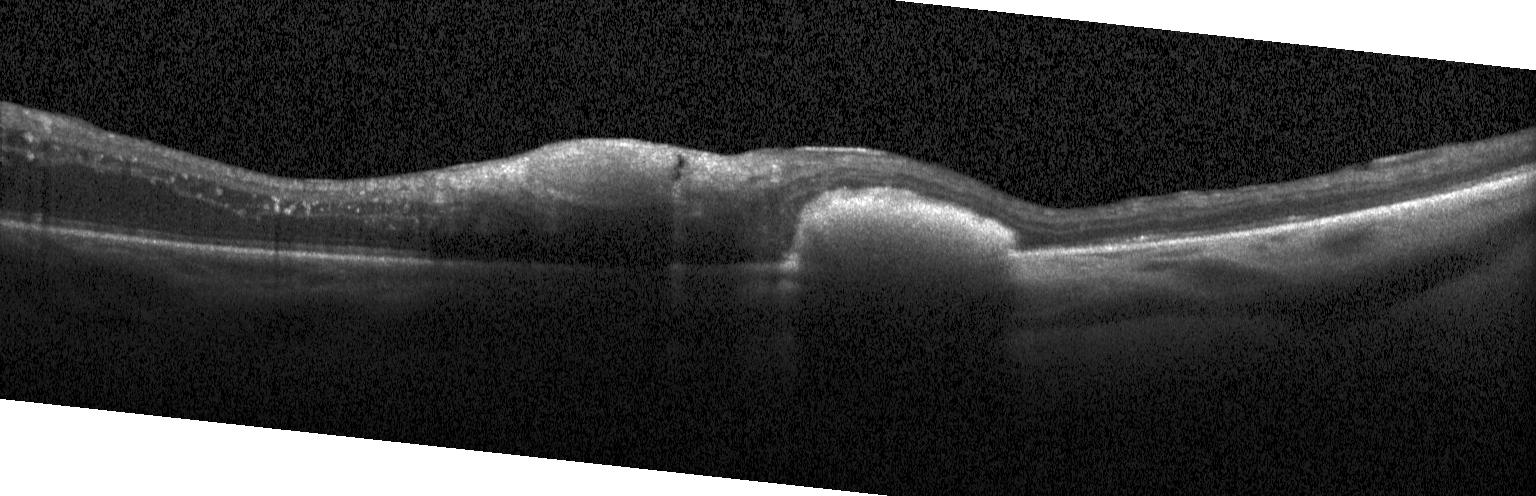

Spectral-domain optical coherence tomography, retinal OCT B-scan, instrument: Heidelberg Spectralis, macular scan — Dx: CNV.